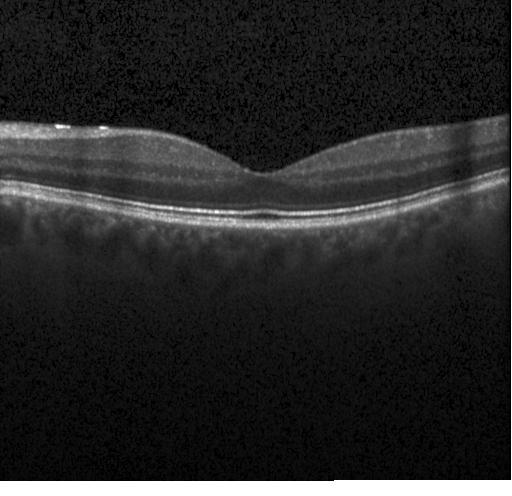
Retinal OCT cross-section, spectral-domain optical coherence tomography — Finding: no CNV, no DME, and no drusen.